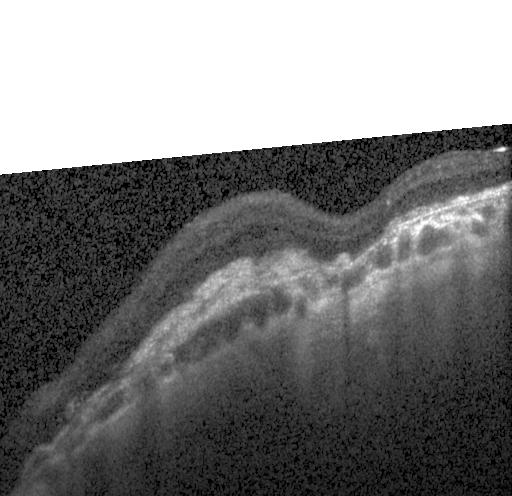 OCT finding: CNV.